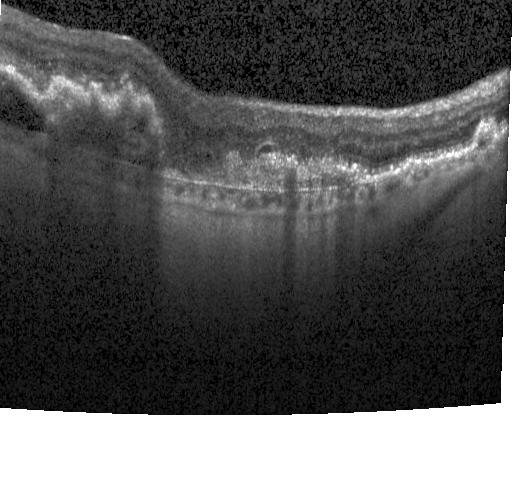

Optical coherence tomography B-scan — Impression: a choroidal neovascular membrane.